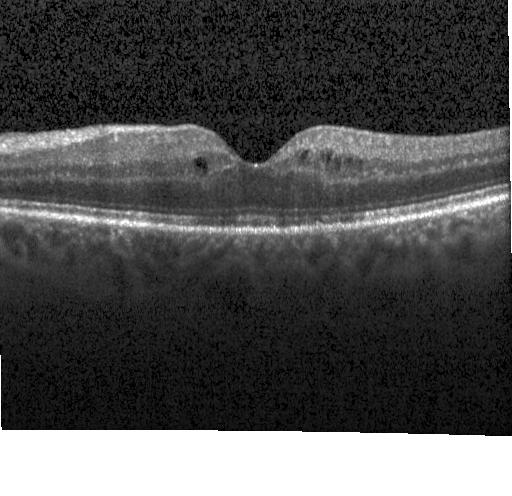 The scan shows diabetic macular edema.